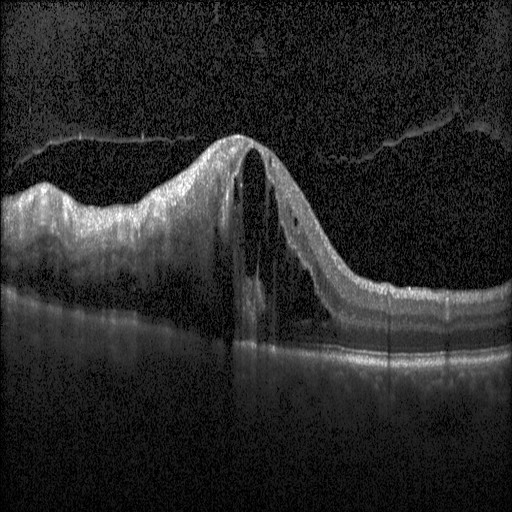
Optical coherence tomography scan; centered on the fovea.
Diabetic macular edema (DME).